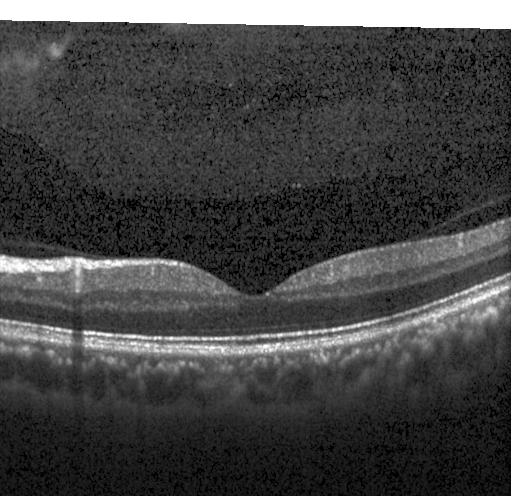 Diagnosis: no CNV, no DME, and no drusen.